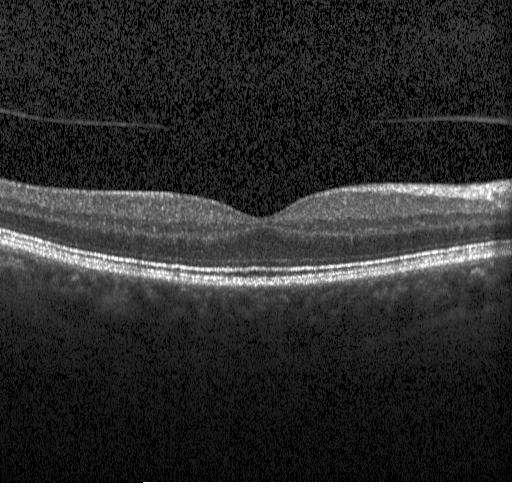
Heidelberg Spectralis OCT system; fovea-centered; OCT B-scan; SD-OCT — Impression: neither choroidal neovascularization, diabetic macular edema, nor drusen.